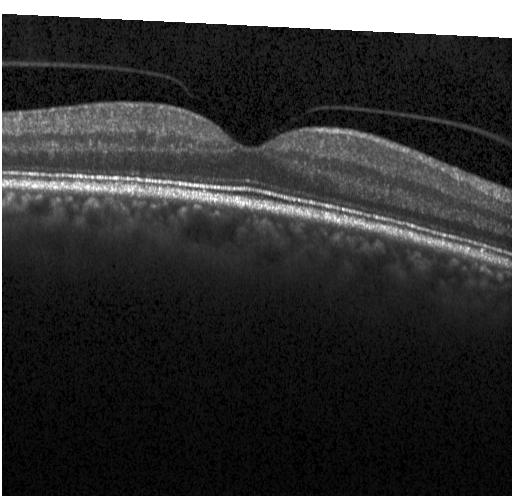 Fovea-centered; retinal OCT B-scan.
Diagnosis: no choroidal neovascularization, diabetic macular edema, or drusen.